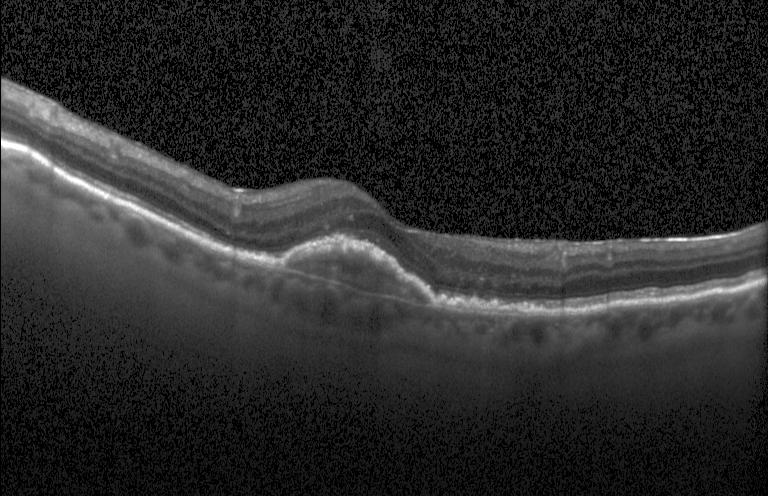 Optical coherence tomography scan
Diagnosis: a choroidal neovascular membrane.